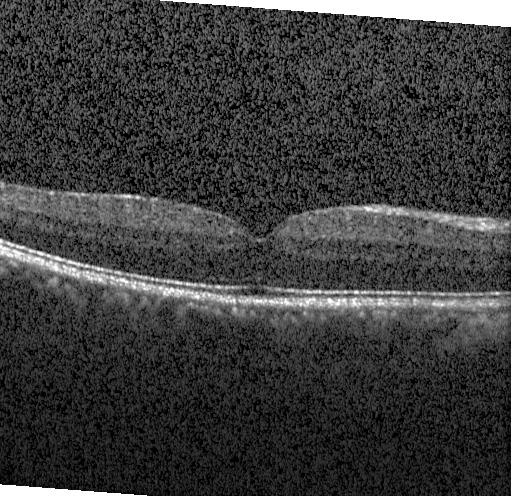 Spectral-domain OCT, OCT B-scan.
Diagnosis: no choroidal neovascularization, diabetic macular edema, or drusen.